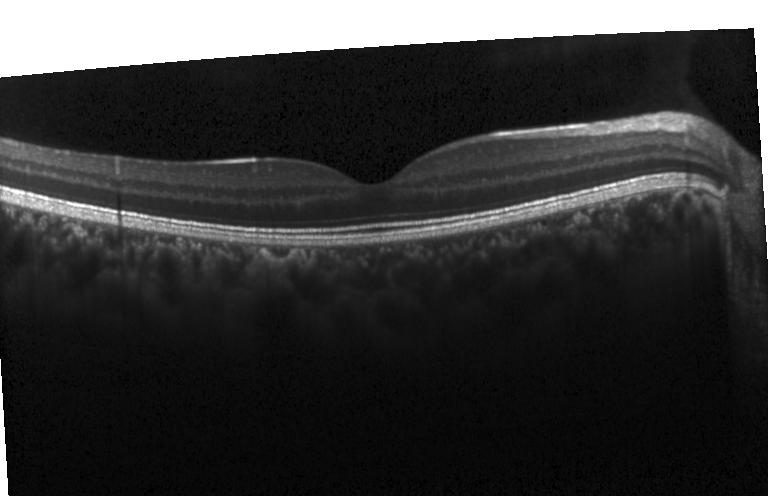 Optical coherence tomography scan
Macular OCT: no choroidal neovascularization, diabetic macular edema, or drusen.